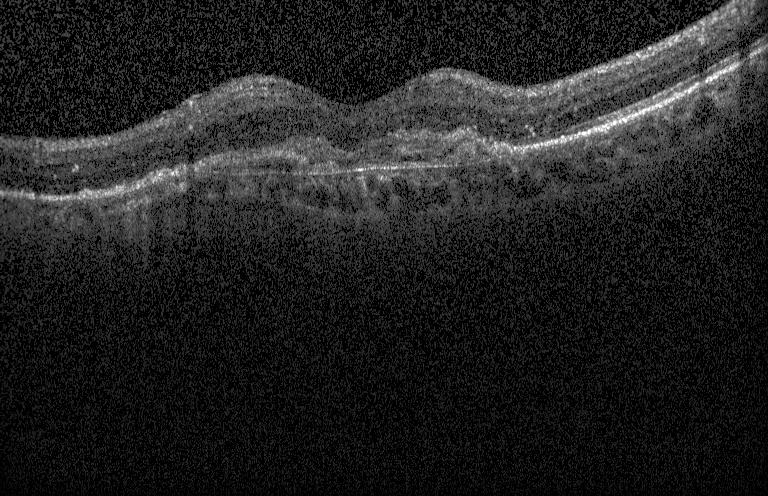

Heidelberg Spectralis OCT system. Spectral-domain optical coherence tomography. Optical coherence tomography B-scan. Through the macula — A choroidal neovascular membrane.